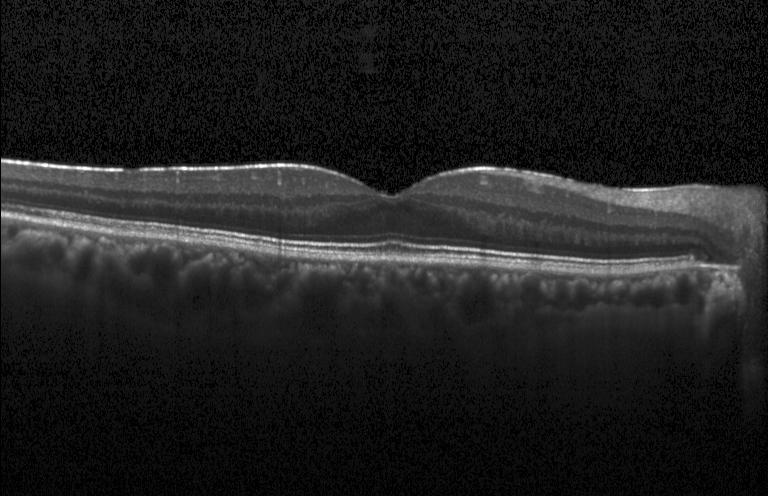
Spectral-domain OCT · retinal OCT B-scan — Diagnosis: no choroidal neovascularization, diabetic macular edema, or drusen.